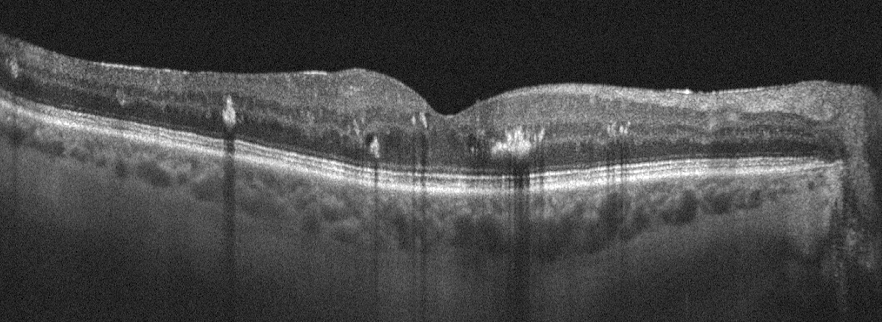

Diagnosis: diabetic macular edema (DME).